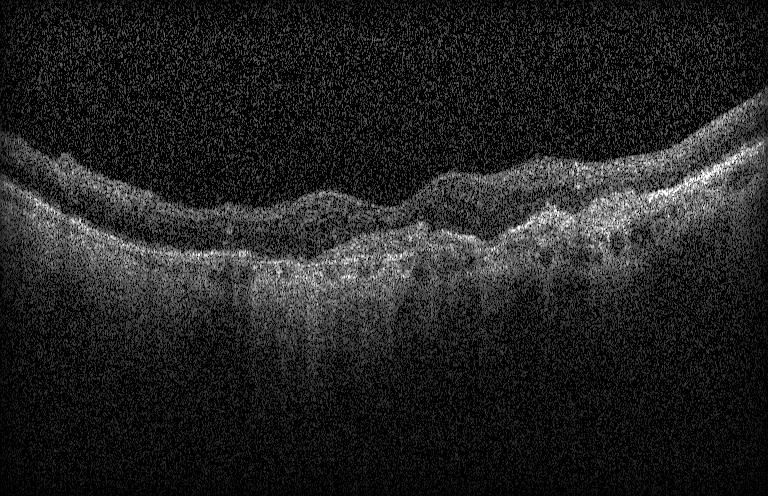

SD-OCT · OCT B-scan · Heidelberg Spectralis OCT system
A choroidal neovascular membrane.